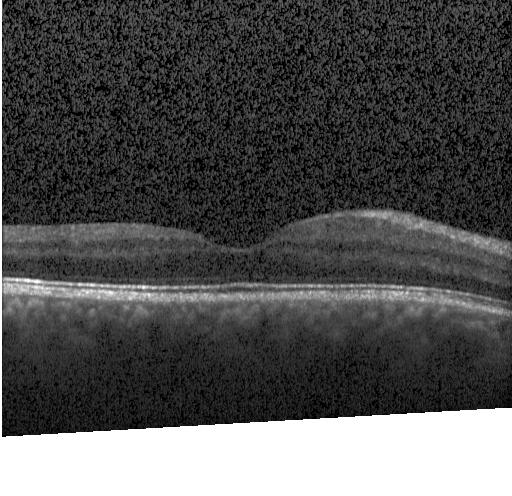

Optical coherence tomography scan — Assessment: neither CNV, DME, nor drusen.